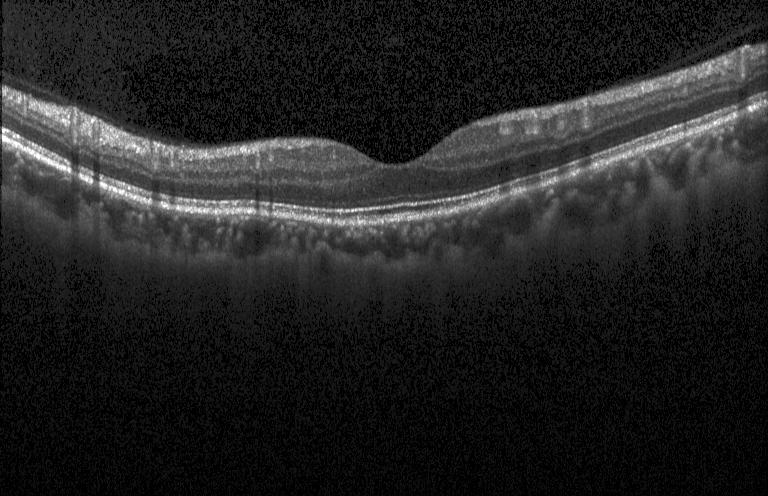

Assessment: no choroidal neovascularization, no diabetic macular edema, and no drusen.